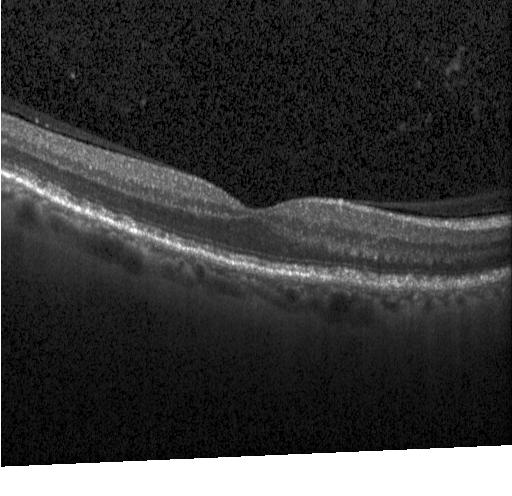
Retinal OCT B-scan; SD-OCT
Finding: no choroidal neovascularization, no diabetic macular edema, and no drusen.